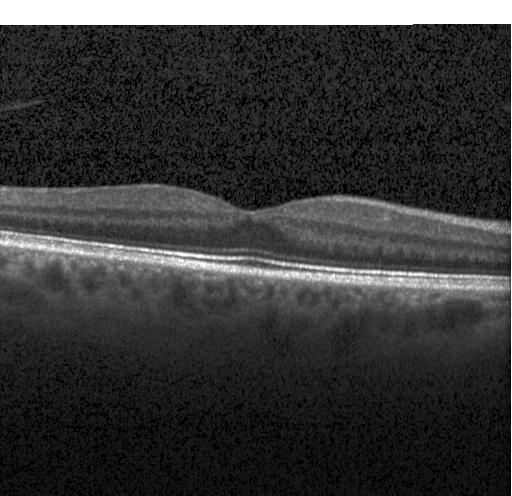

Centered on the fovea; optical coherence tomography B-scan; SD-OCT. No CNV, no DME, and no drusen.